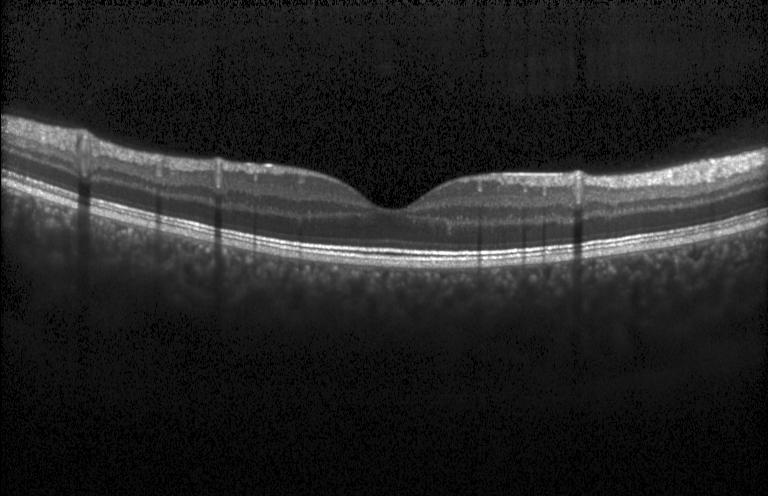

Horizontal scan through the fovea, optical coherence tomography scan, spectral-domain optical coherence tomography.
Finding: no choroidal neovascularization, no diabetic macular edema, and no drusen.